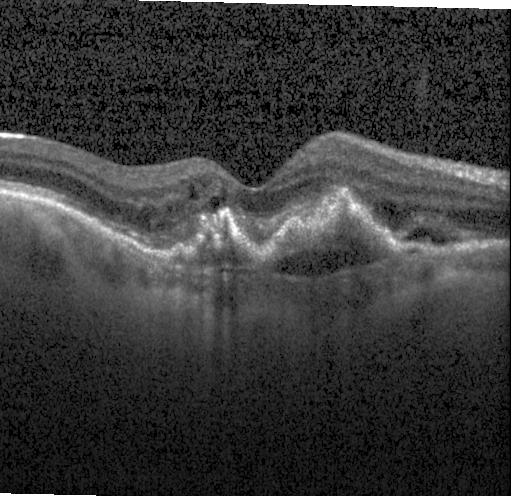 Assessment: a choroidal neovascular membrane.